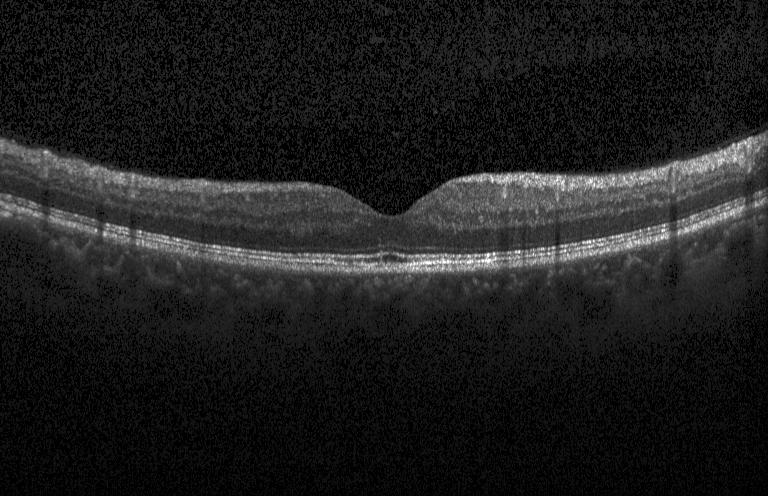 Through the macula · acquired on a Heidelberg Spectralis · spectral-domain optical coherence tomography · optical coherence tomography scan — Diagnosis: neither choroidal neovascularization, diabetic macular edema, nor drusen.